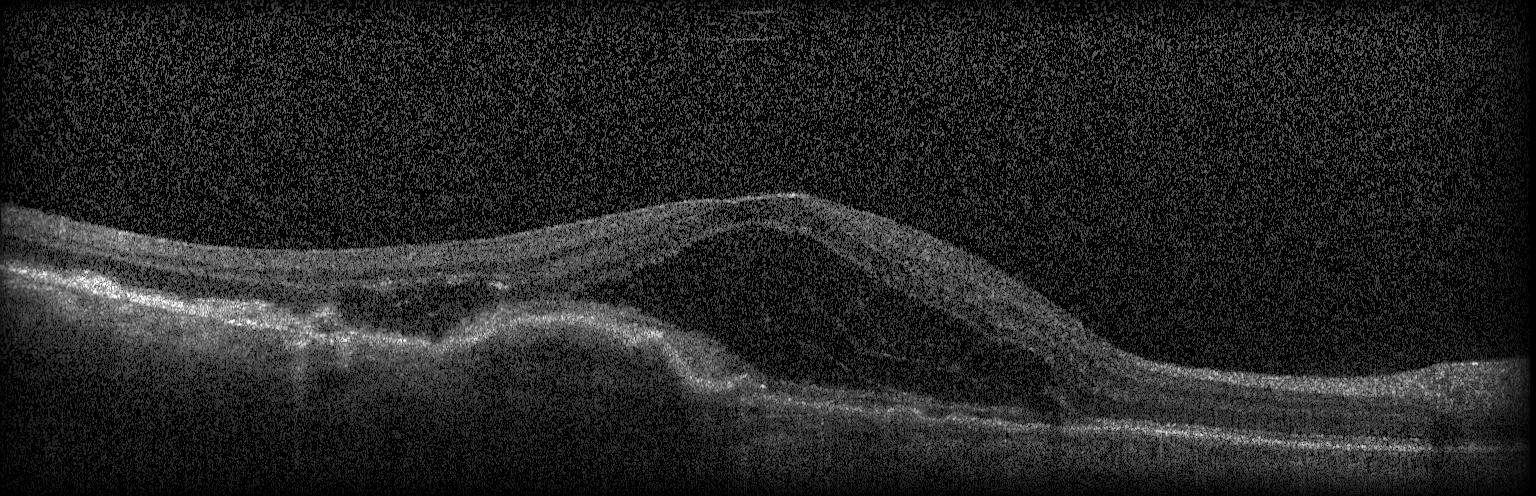
Impression: a choroidal neovascular membrane.